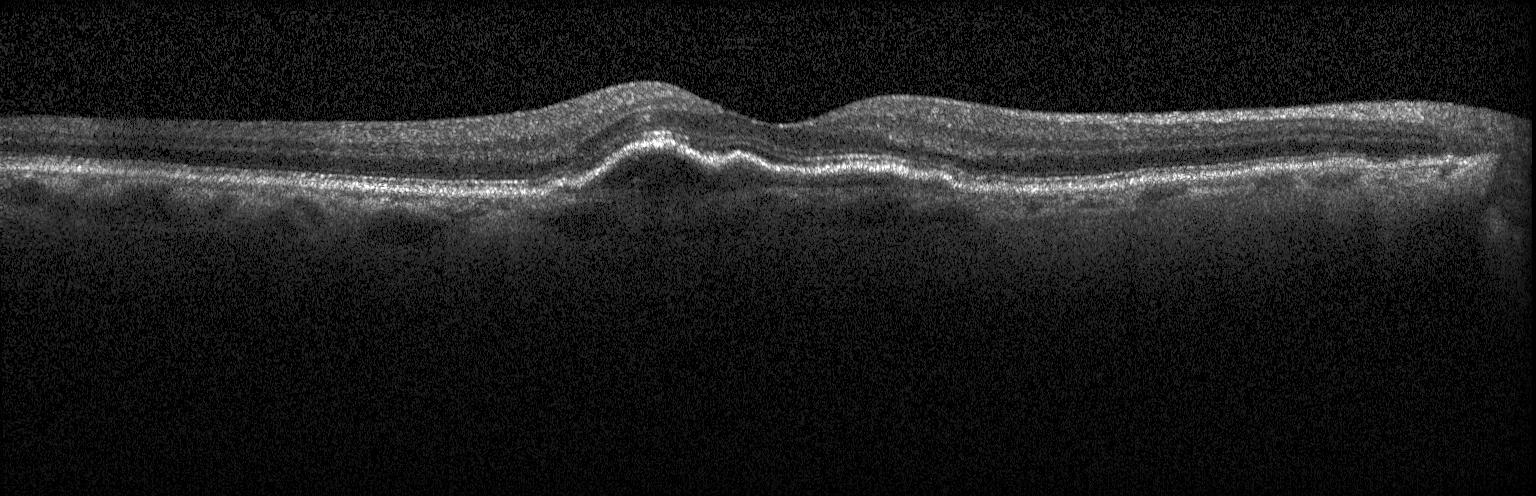 Spectral-domain OCT B-scan: choroidal neovascularization (CNV).